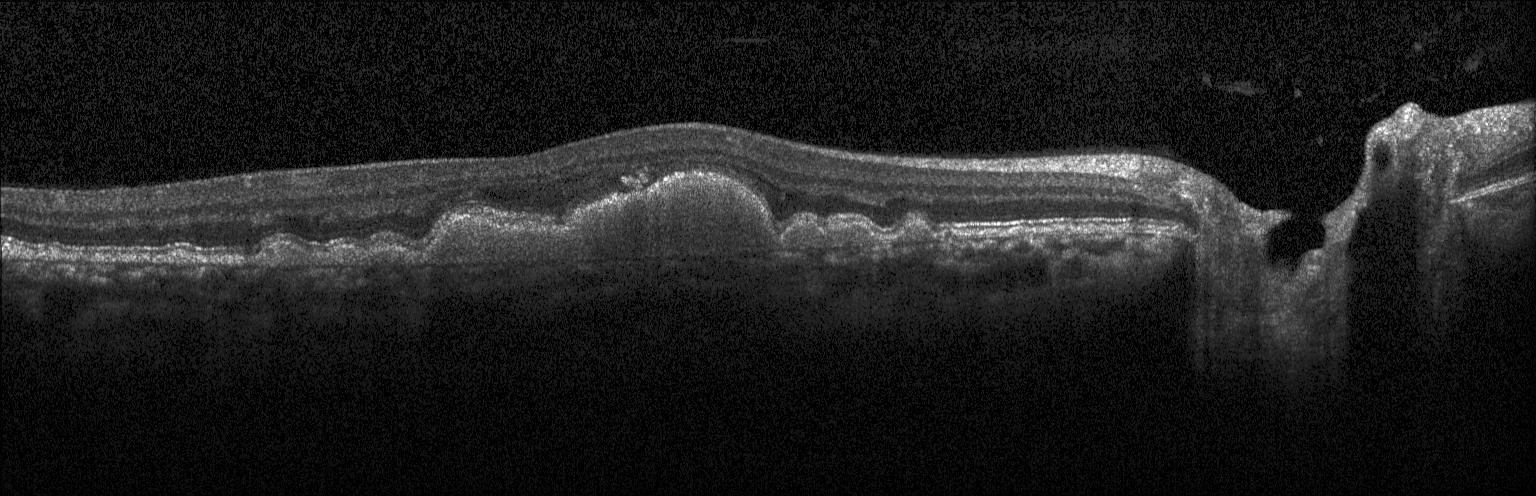
Sub-RPE drusenoid deposits.